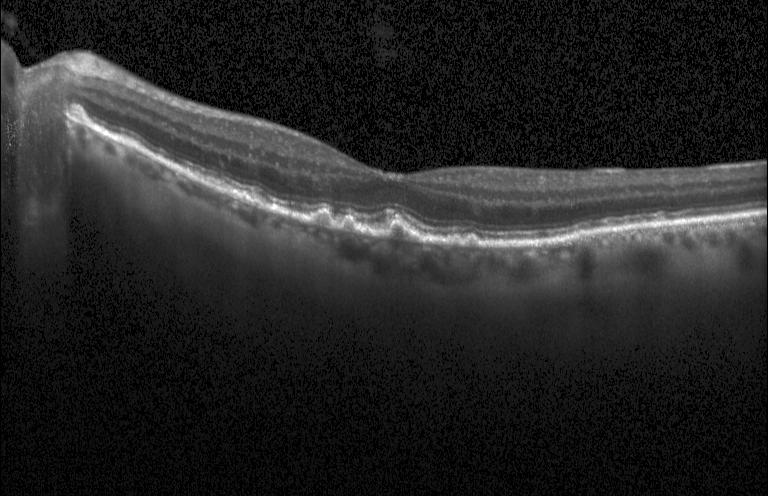

OCT line scan. SD-OCT. Horizontal scan through the fovea. Heidelberg Spectralis OCT system. Diagnosis: multiple drusen.